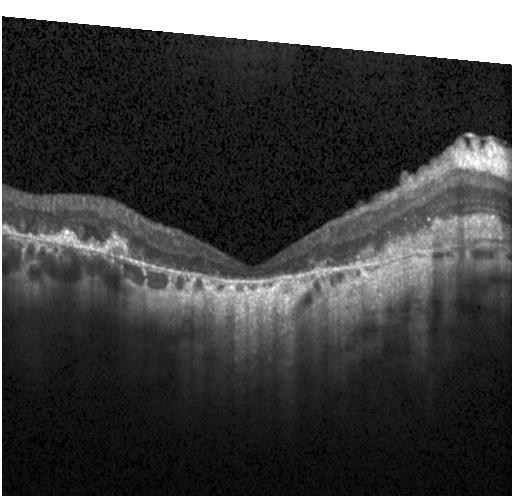
Optical coherence tomography B-scan; Heidelberg Spectralis; fovea-centered. Impression: a choroidal neovascular membrane.